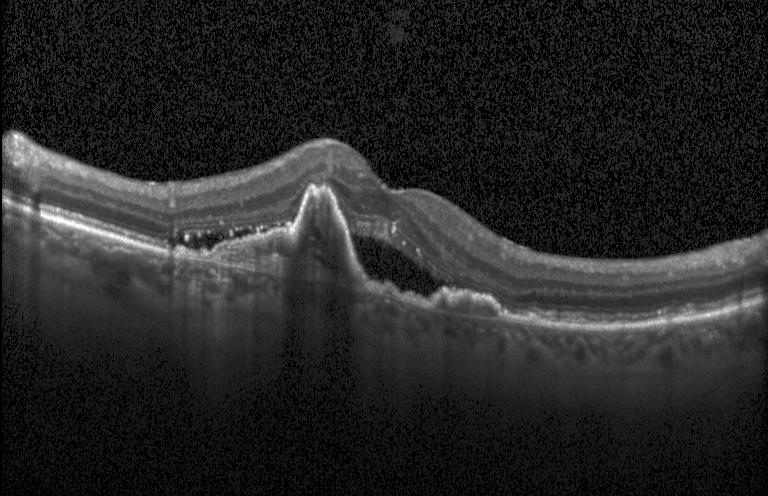

Retinal OCT B-scan · fovea-centered. Diagnosis: a choroidal neovascular membrane.